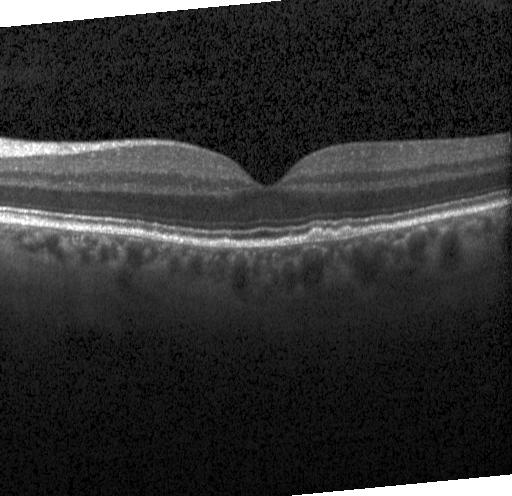 Finding: drusen.